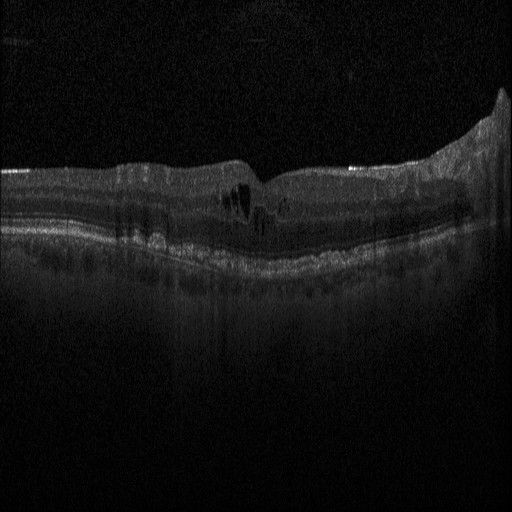 Through the macula, optical coherence tomography B-scan. DME.